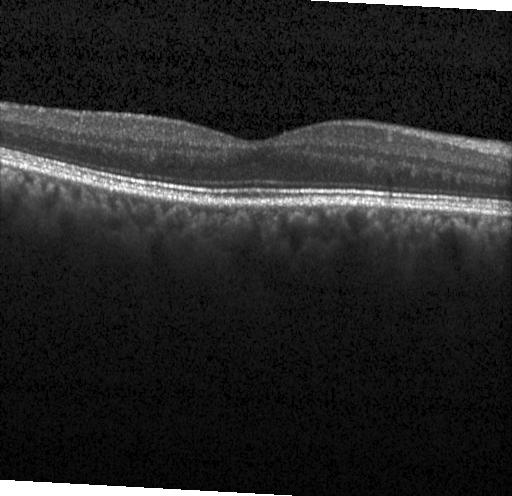
Through the macula; optical coherence tomography B-scan
Assessment: neither choroidal neovascularization, diabetic macular edema, nor drusen.